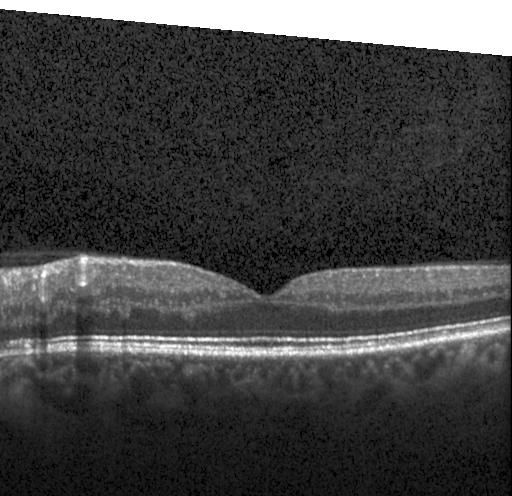
Diagnosis: neither choroidal neovascularization, diabetic macular edema, nor drusen.